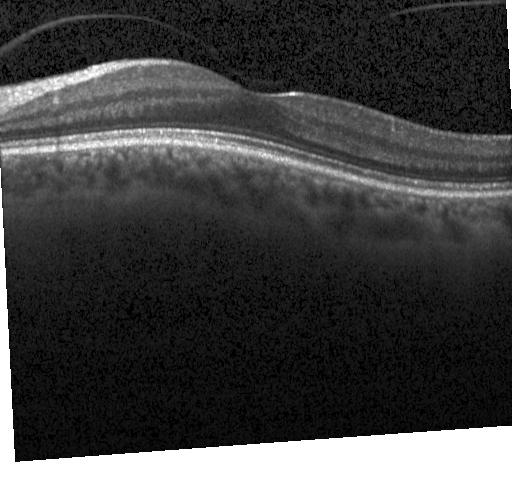

Retinal OCT cross-section; SD-OCT
The scan shows no evidence of choroidal neovascularization, diabetic macular edema, or drusen.